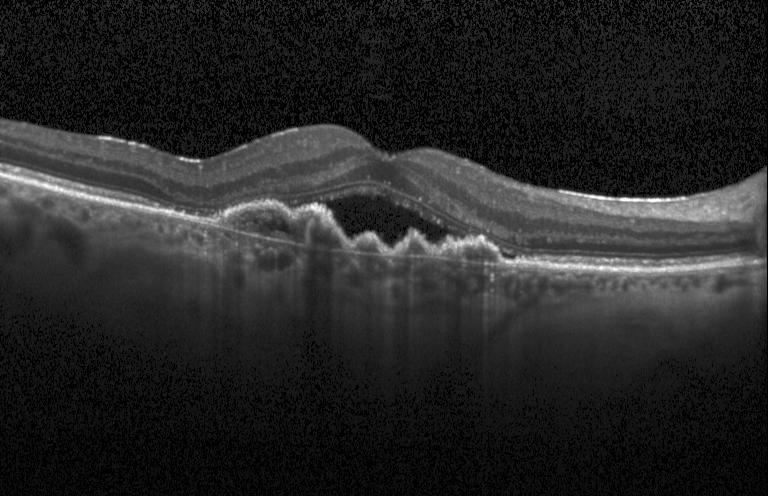

Retinal OCT B-scan.
Impression: choroidal neovascularization (CNV).